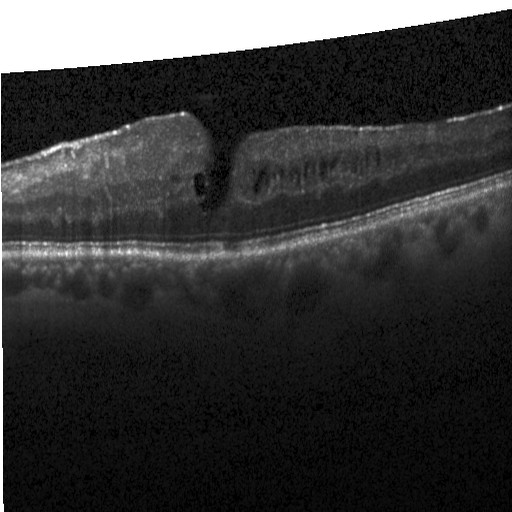 SD-OCT. Retinal OCT B-scan. This B-scan demonstrates diabetic macular edema (DME).